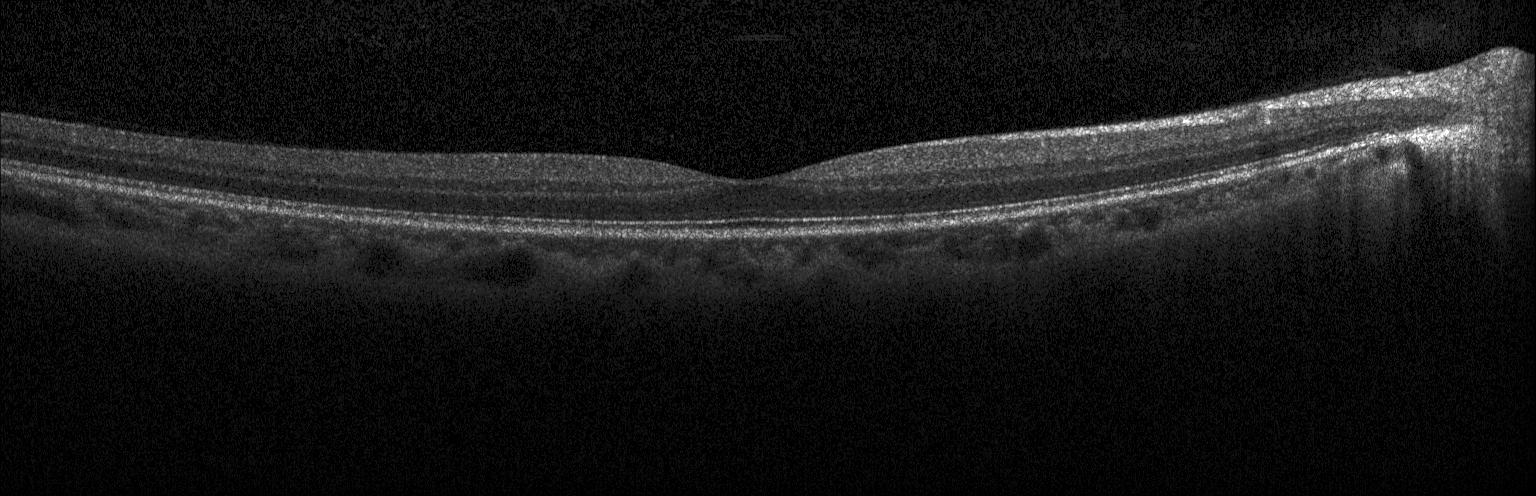
Spectral-domain OCT B-scan: no choroidal neovascularization, no diabetic macular edema, and no drusen.